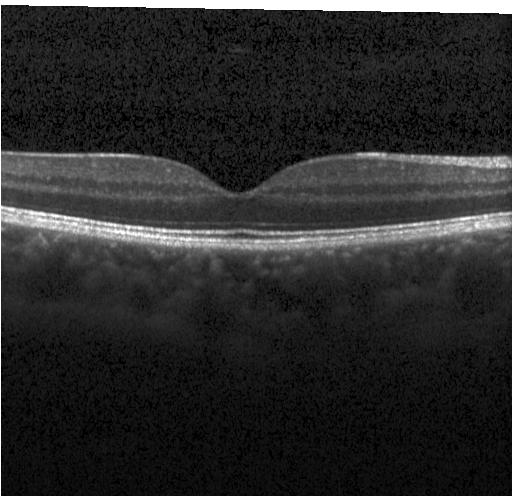 Retinal OCT B-scan, Heidelberg Spectralis, spectral-domain optical coherence tomography.
Impression: no choroidal neovascularization, no diabetic macular edema, and no drusen.